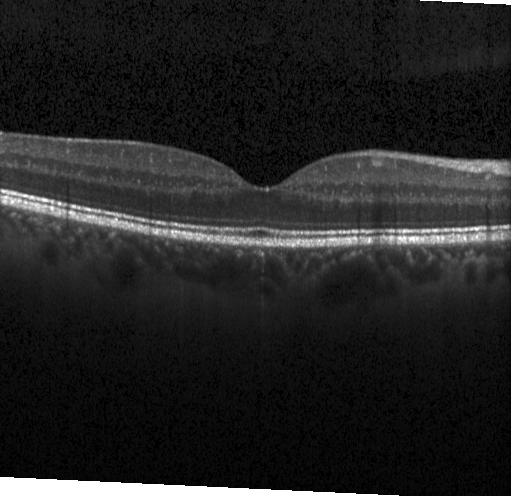

Spectral-domain optical coherence tomography, instrument: Heidelberg Spectralis, retinal OCT cross-section.
Impression: neither choroidal neovascularization, diabetic macular edema, nor drusen.